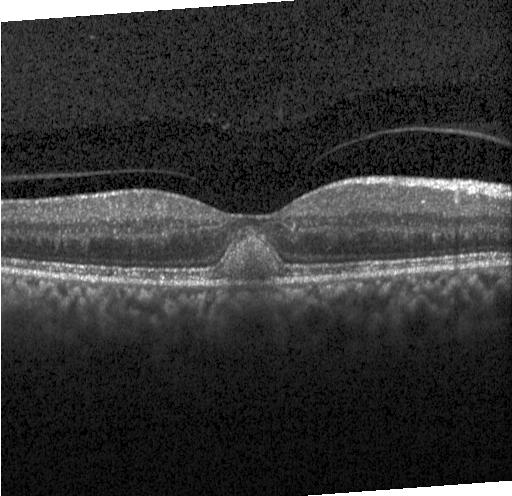

Optical coherence tomography B-scan.
Impression: a choroidal neovascular membrane.